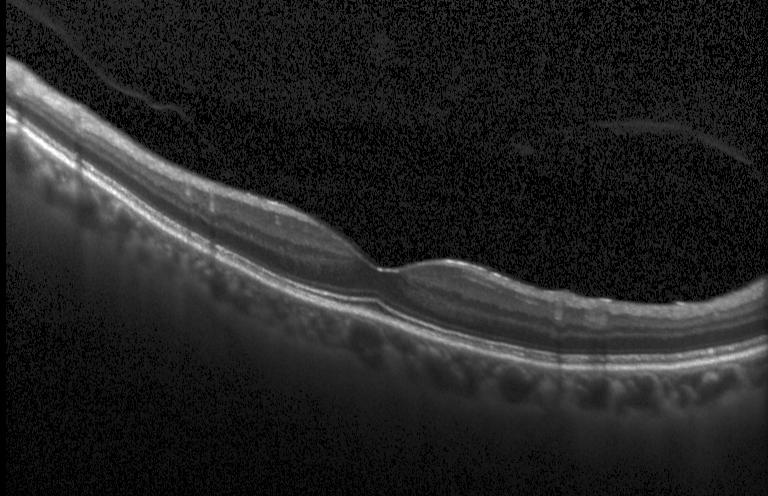

OCT line scan — The scan shows neither choroidal neovascularization, diabetic macular edema, nor drusen.